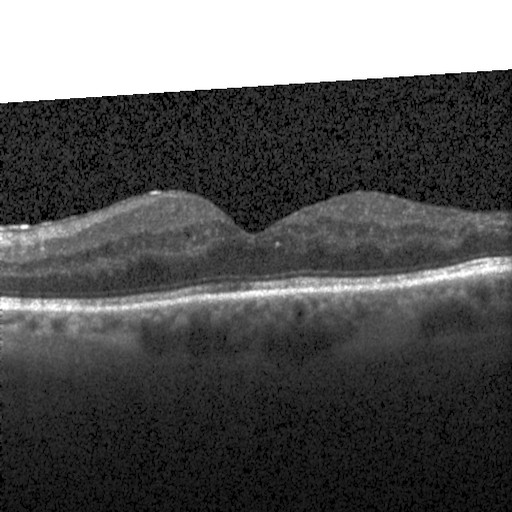 Optical coherence tomography scan.
Impression: diabetic macular edema (DME).